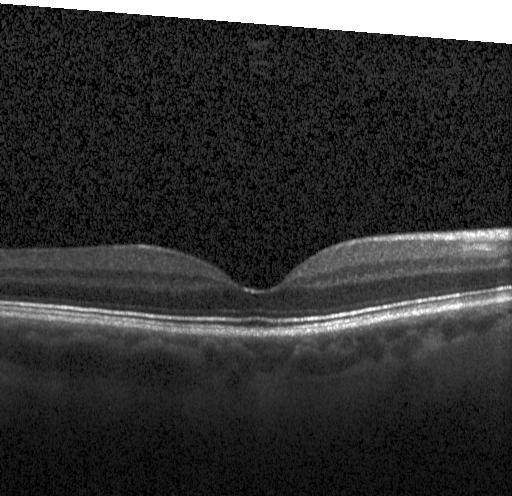 Macular OCT: no evidence of CNV, DME, or drusen.